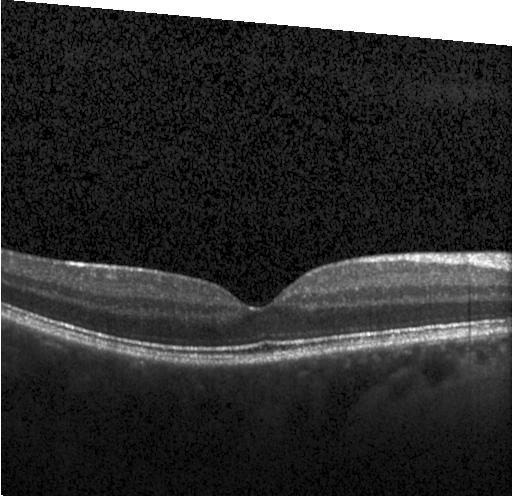

Optical coherence tomography B-scan. Heidelberg Spectralis. Spectral-domain OCT.
This B-scan demonstrates no choroidal neovascularization, no diabetic macular edema, and no drusen.